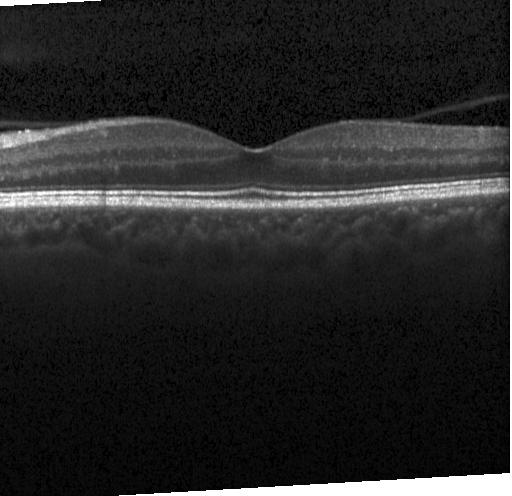
Optical coherence tomography scan; SD-OCT; macular scan — The scan shows neither CNV, DME, nor drusen.